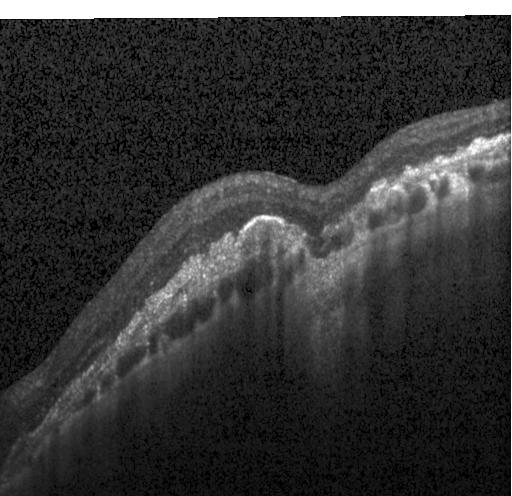 Spectral-domain OCT; through the macula; OCT B-scan; acquired on a Heidelberg Spectralis
Finding: a choroidal neovascular membrane.